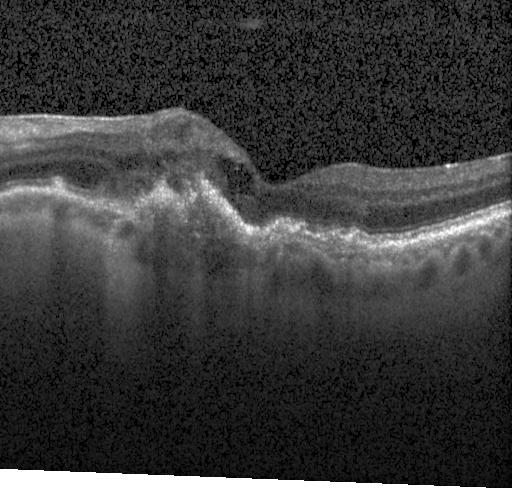

Retinal OCT cross-section showing a choroidal neovascular membrane.